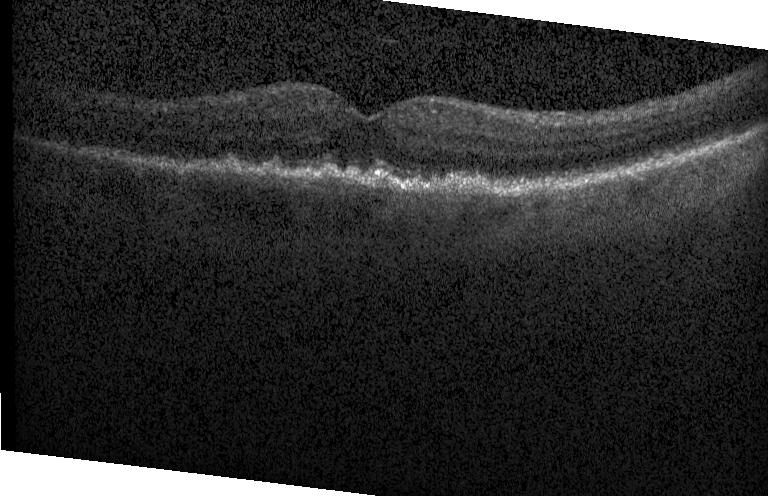
Optical coherence tomography B-scan
Impression: drusen.